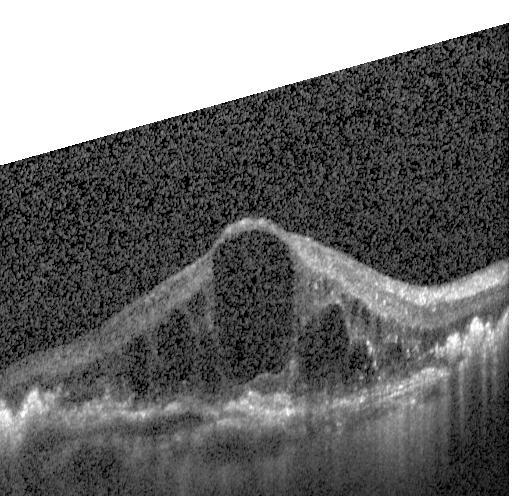
Optical coherence tomography B-scan.
This B-scan demonstrates a choroidal neovascular membrane.